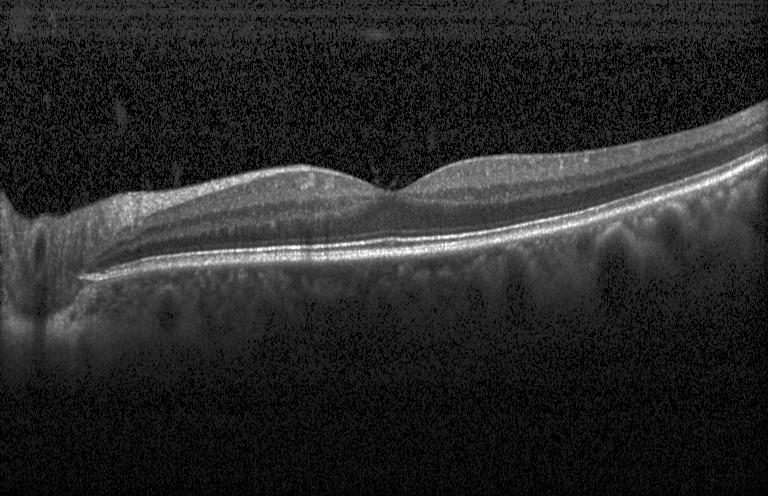
Macular OCT: no choroidal neovascularization, no diabetic macular edema, and no drusen.